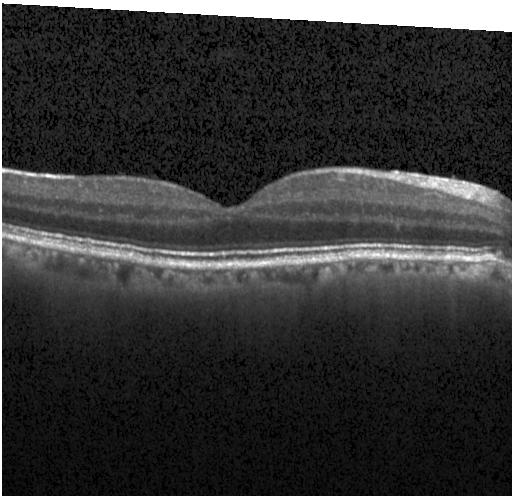 Retinal OCT cross-section
Finding: no evidence of choroidal neovascularization, diabetic macular edema, or drusen.